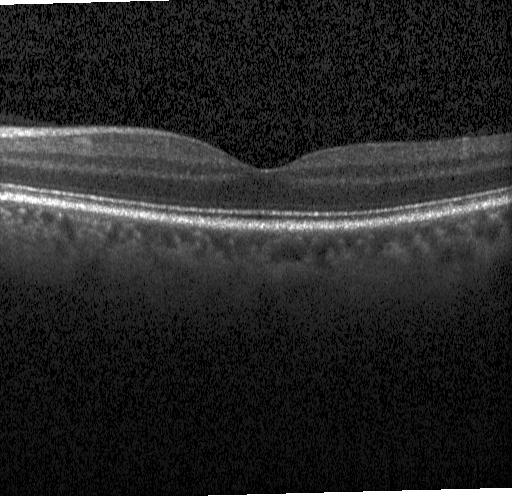 OCT line scan.
OCT finding: no CNV, no DME, and no drusen.